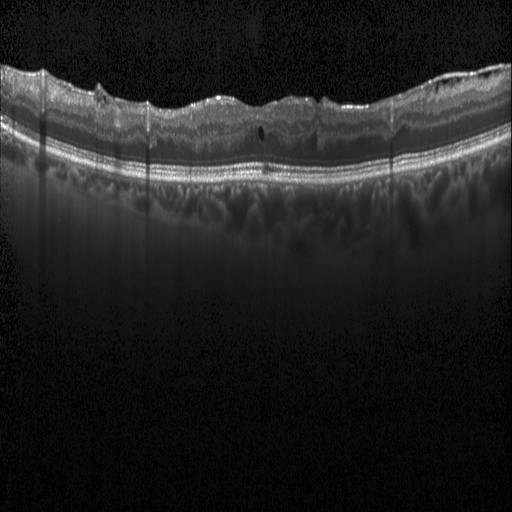

Impression: diabetic macular edema.